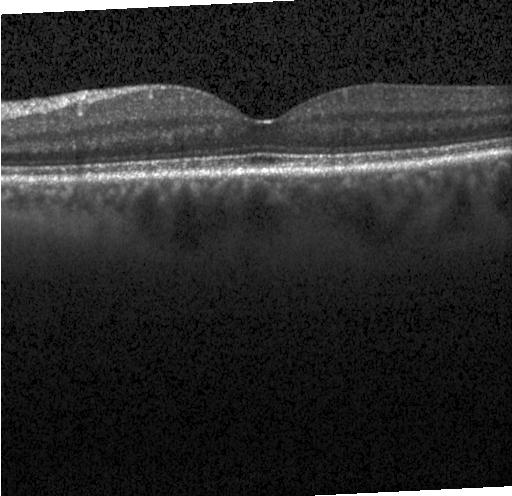

Diagnosis: no choroidal neovascularization, no diabetic macular edema, and no drusen.